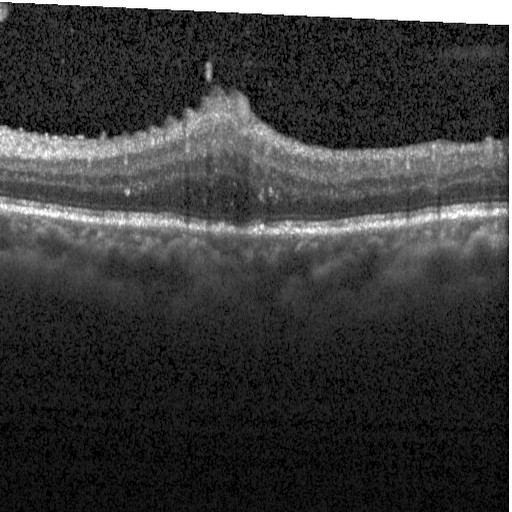
Fovea-centered; optical coherence tomography B-scan; spectral-domain optical coherence tomography; instrument: Heidelberg Spectralis.
Finding: DME.